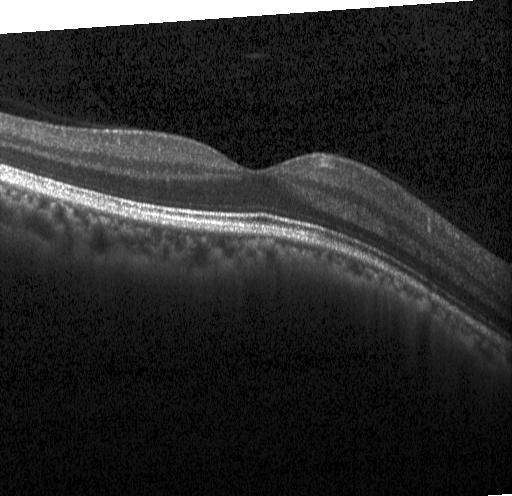
OCT line scan.
OCT finding: no CNV, no DME, and no drusen.